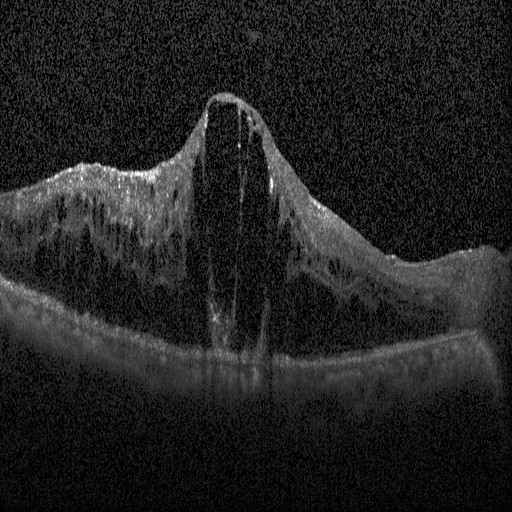 Retinal OCT cross-section showing DME.